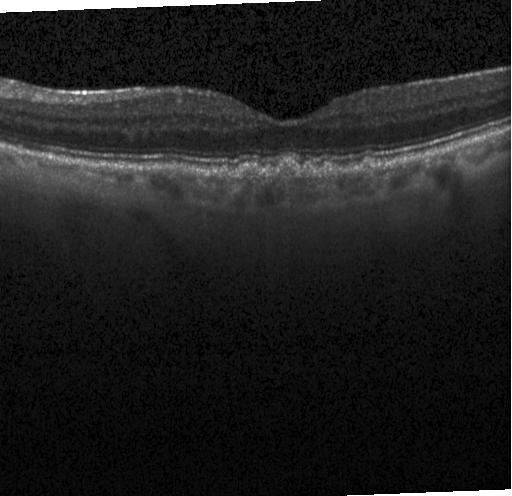
Macular OCT demonstrating drusen.